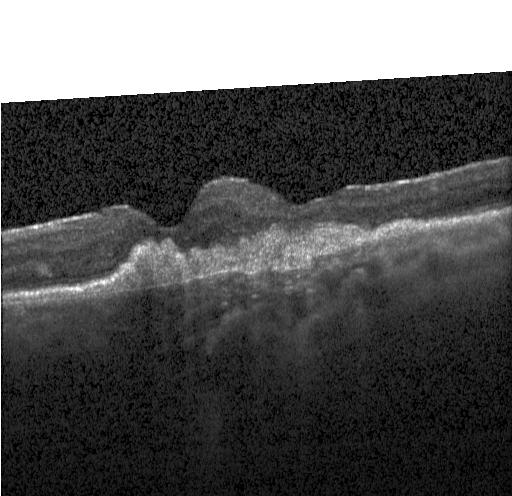 OCT B-scan. Choroidal neovascularization (CNV).